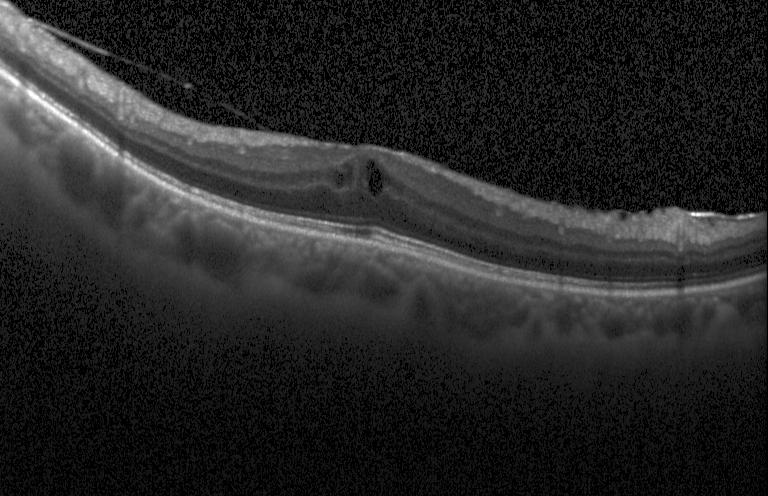

Spectral-domain OCT. Heidelberg Spectralis OCT system. Optical coherence tomography scan. Centered on the fovea.
Assessment: diabetic macular edema.